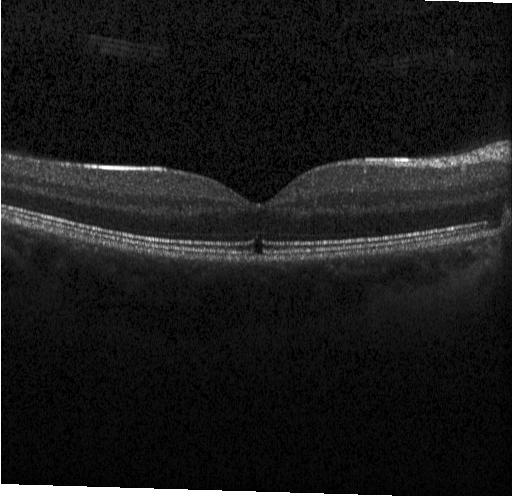

Retinal OCT B-scan.
Finding: no CNV, no DME, and no drusen.